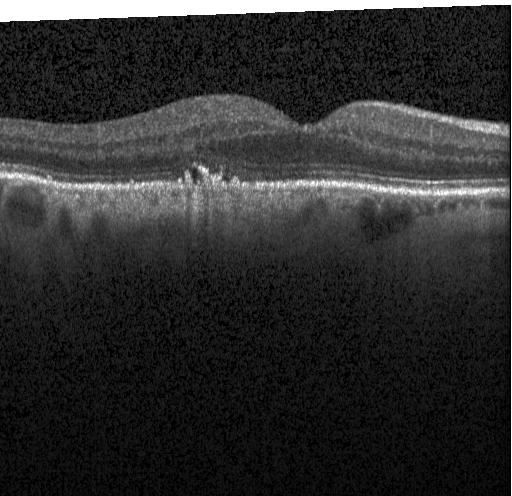
Optical coherence tomography B-scan — Diagnosis: a choroidal neovascular membrane.